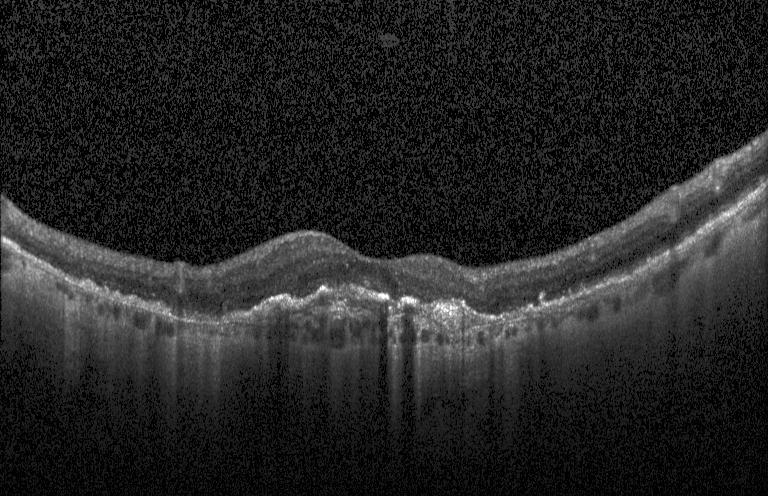
OCT B-scan
The scan shows a choroidal neovascular membrane.